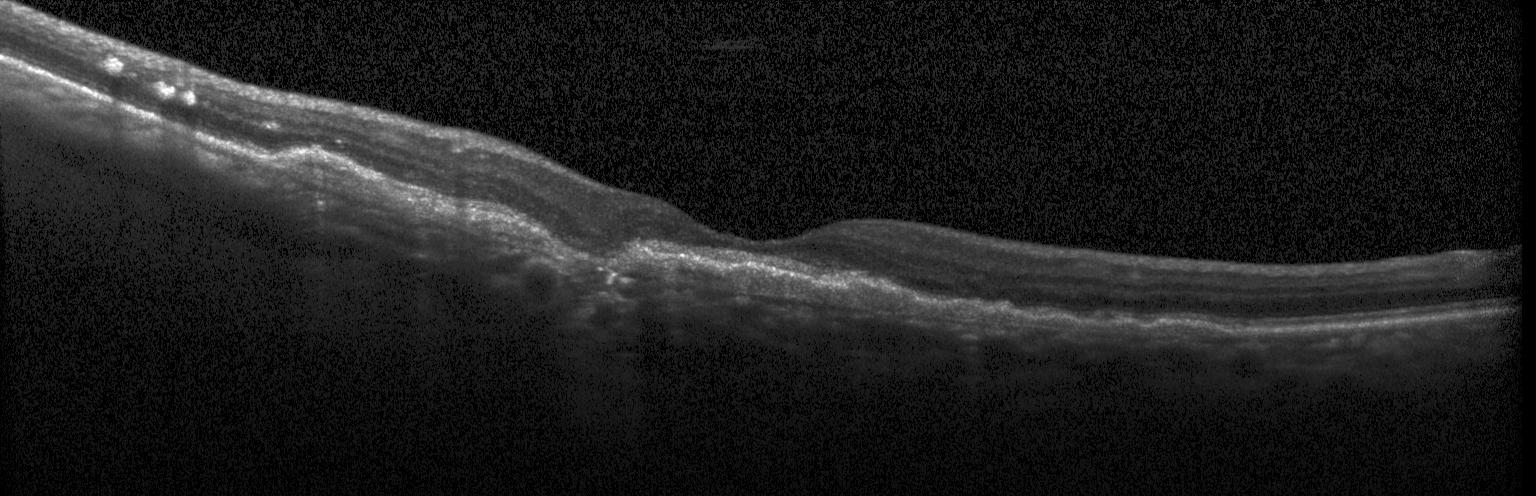

Retinal OCT B-scan; spectral-domain OCT; through the macula. This B-scan demonstrates a choroidal neovascular membrane.